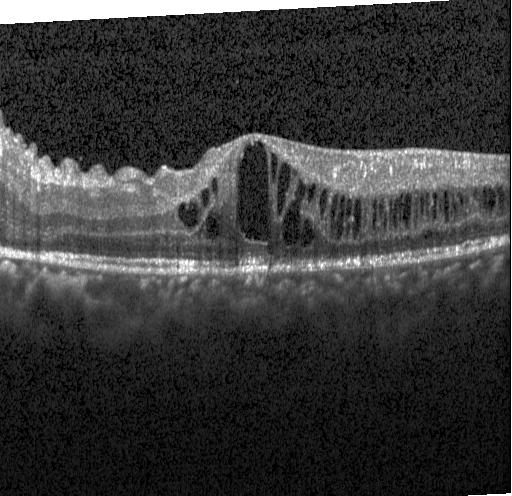 The scan shows diabetic macular edema (DME).